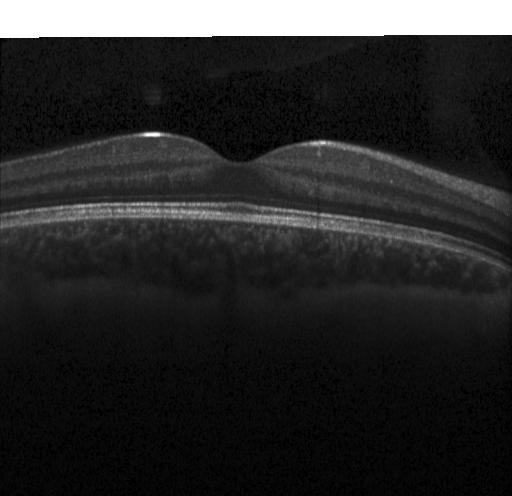

OCT B-scan
Diagnosis: no evidence of CNV, DME, or drusen.